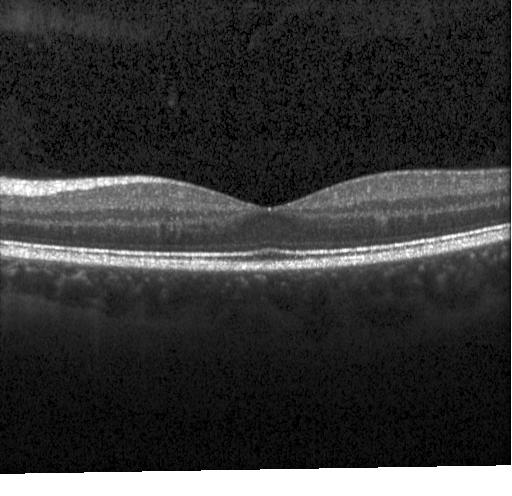 Spectral-domain OCT B-scan: neither choroidal neovascularization, diabetic macular edema, nor drusen.